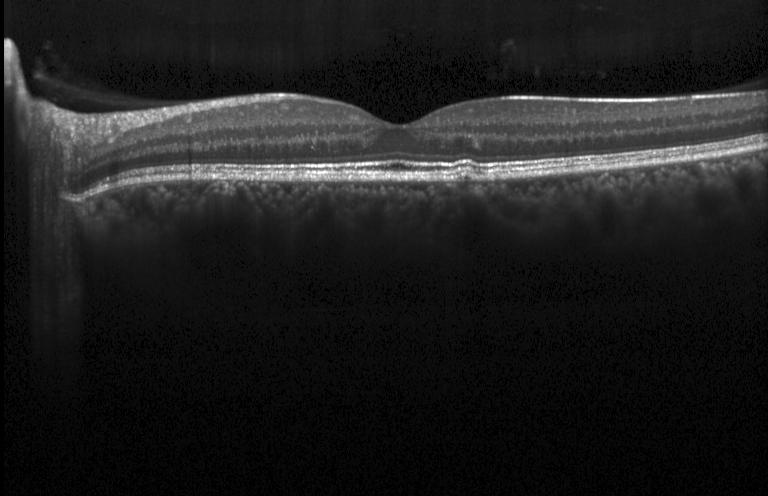 This B-scan demonstrates multiple drusen.